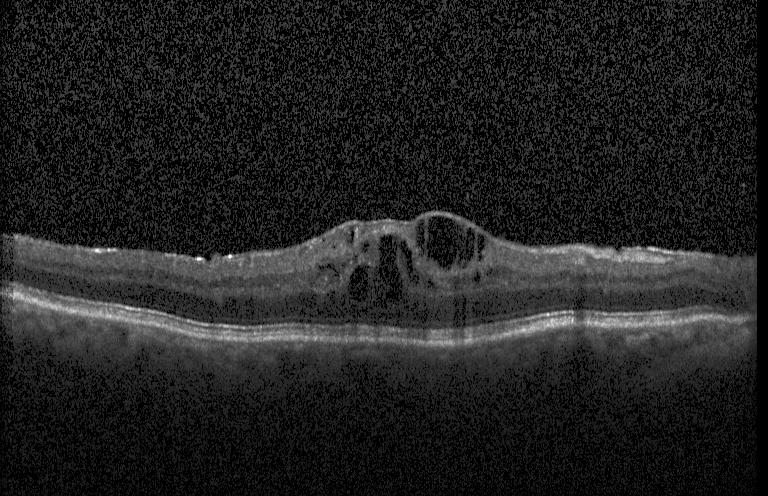
OCT B-scan
Diagnosis: DME.